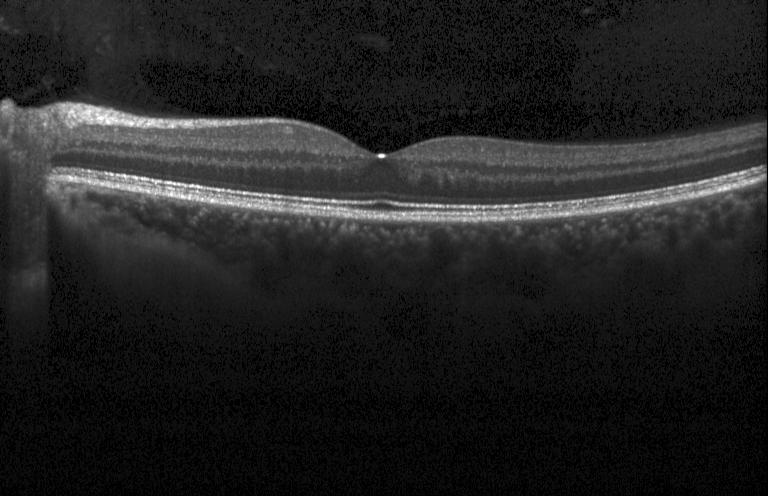

Retinal OCT cross-section; Heidelberg Spectralis
Diagnosis: no choroidal neovascularization, no diabetic macular edema, and no drusen.